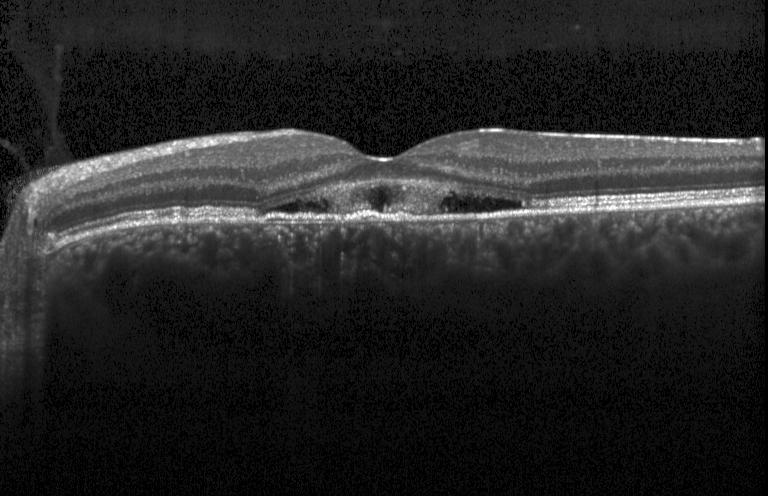 Heidelberg Spectralis · OCT line scan · spectral-domain optical coherence tomography · through the macula. Macular OCT: choroidal neovascularization.